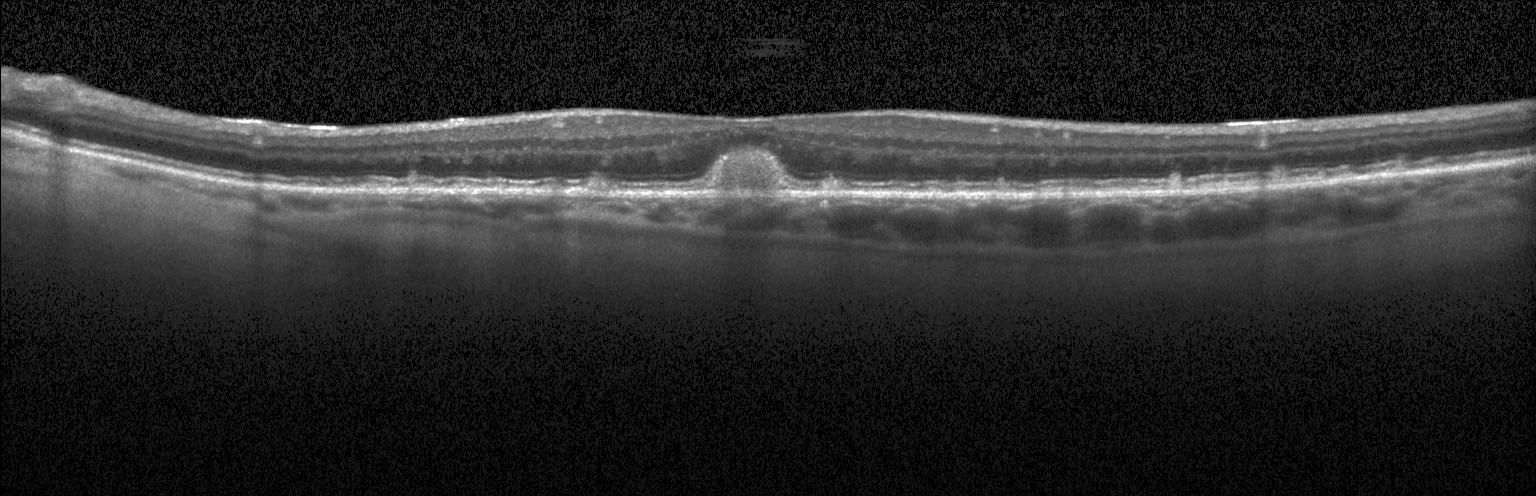

Impression: a choroidal neovascular membrane.